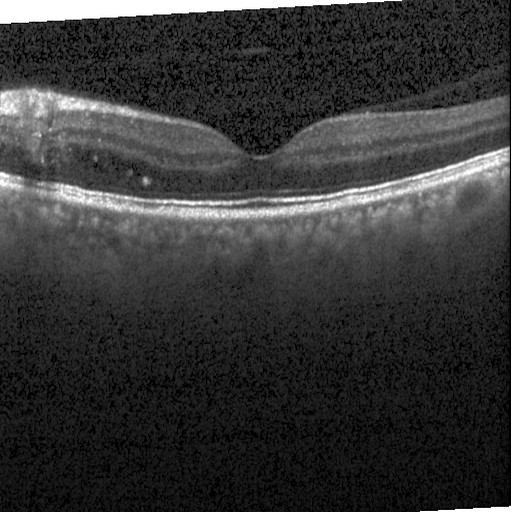 Optical coherence tomography B-scan
DME.